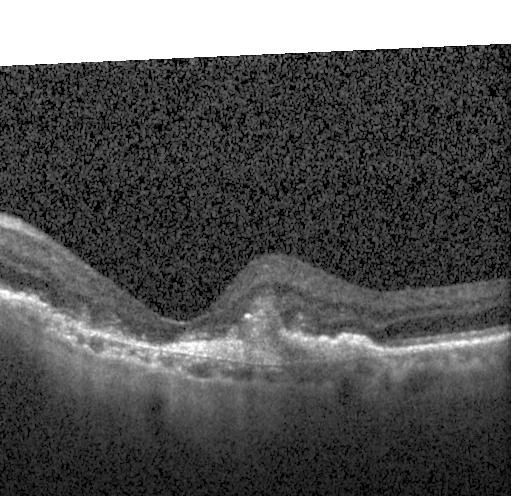 Optical coherence tomography scan
Diagnosis: choroidal neovascularization.